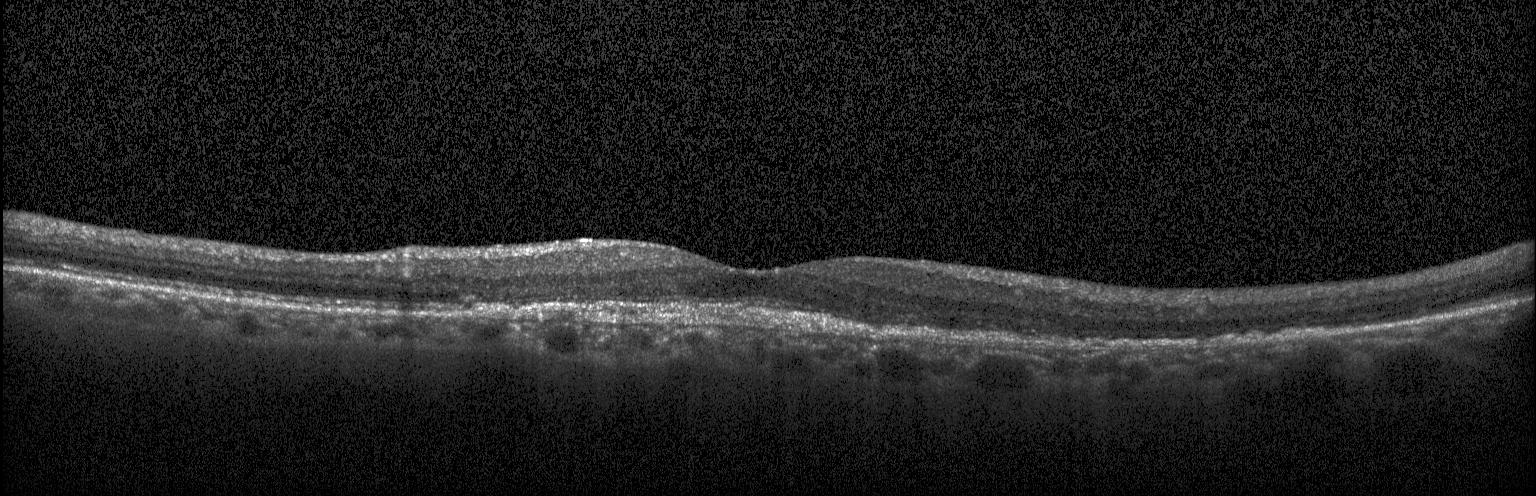 Fovea-centered · OCT line scan · Heidelberg Spectralis OCT system · spectral-domain optical coherence tomography — This B-scan demonstrates choroidal neovascularization (CNV).